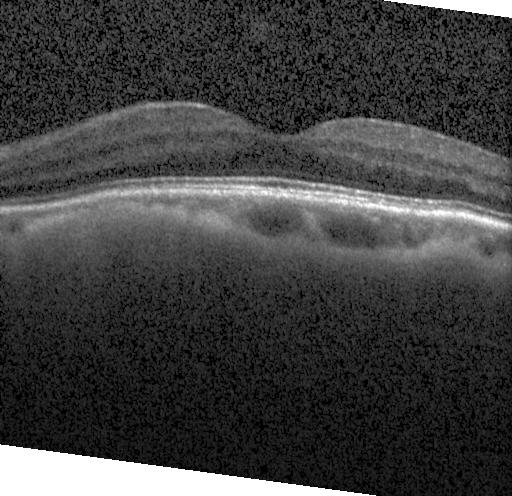
Diagnosis: no evidence of choroidal neovascularization, diabetic macular edema, or drusen.